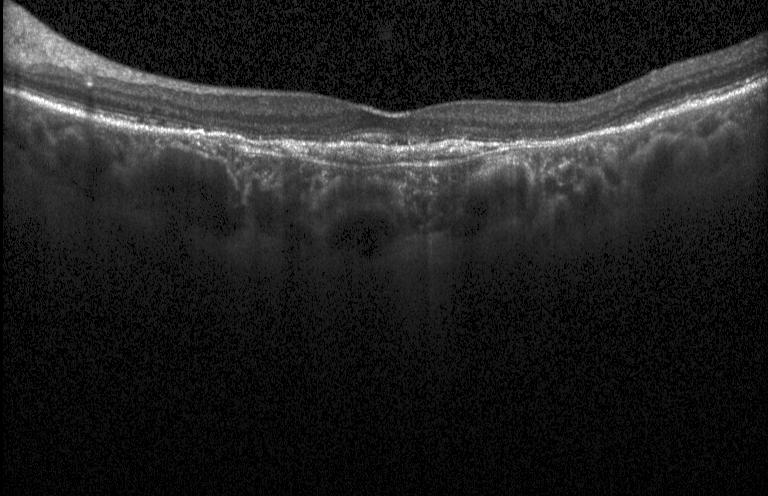 SD-OCT. Macular scan. Instrument: Heidelberg Spectralis. Retinal OCT cross-section. Assessment: choroidal neovascularization (CNV).